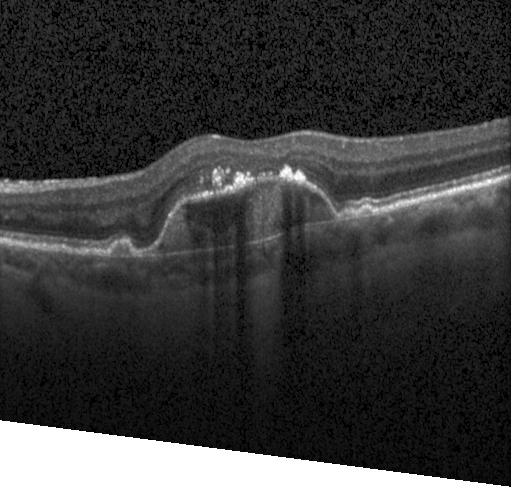 Fovea-centered. OCT B-scan. Spectral-domain OCT. Heidelberg Spectralis OCT system — Impression: CNV.